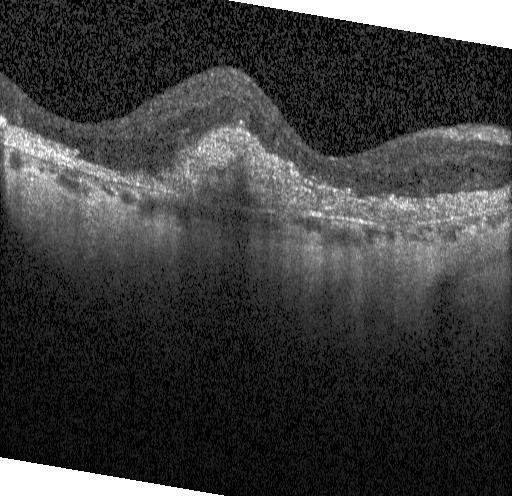

OCT scan showing a choroidal neovascular membrane.